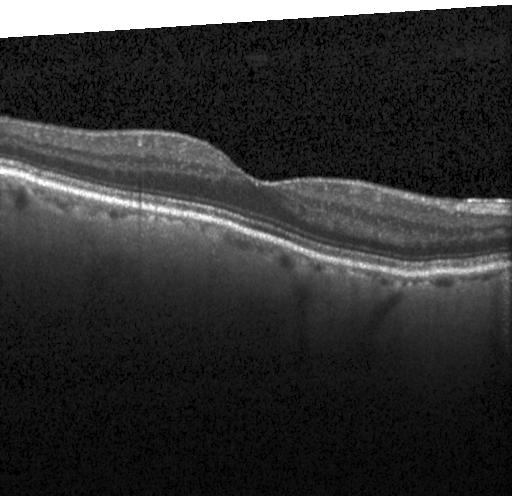
Macular scan, Heidelberg Spectralis OCT system, spectral-domain OCT, OCT line scan.
Dx: no CNV, DME, or drusen.